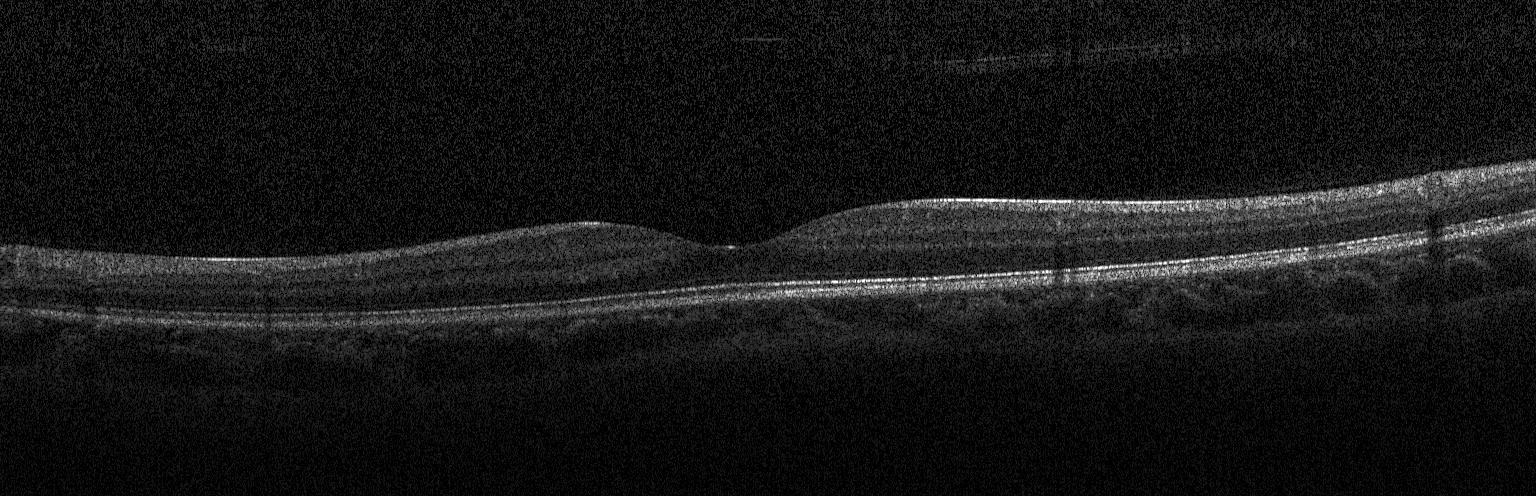
OCT scan showing no evidence of choroidal neovascularization, diabetic macular edema, or drusen.